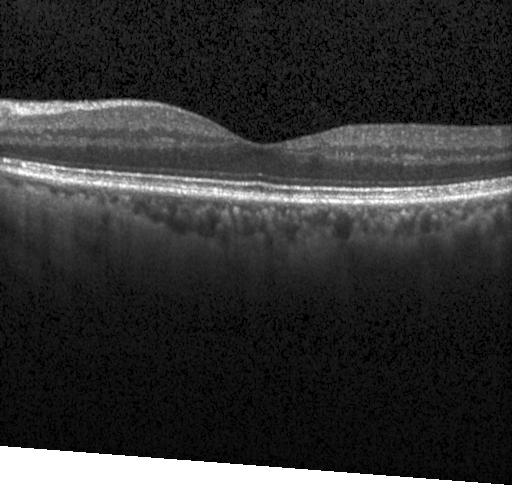

Diagnosis: neither choroidal neovascularization, diabetic macular edema, nor drusen.